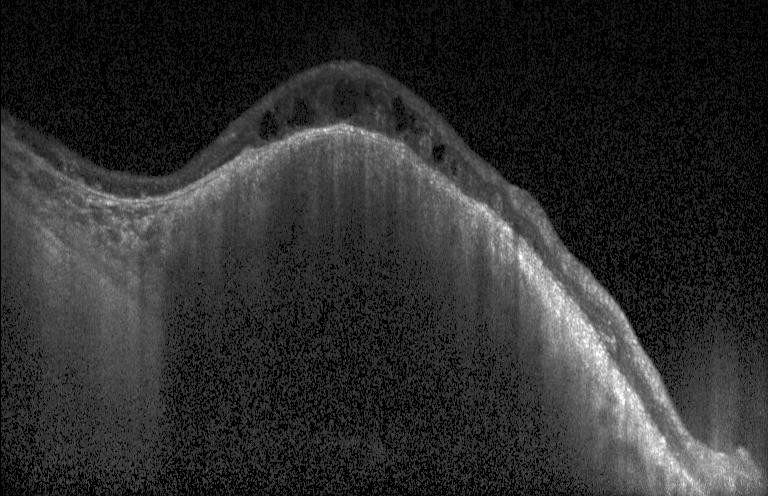

Diagnosis: diabetic macular edema (DME).